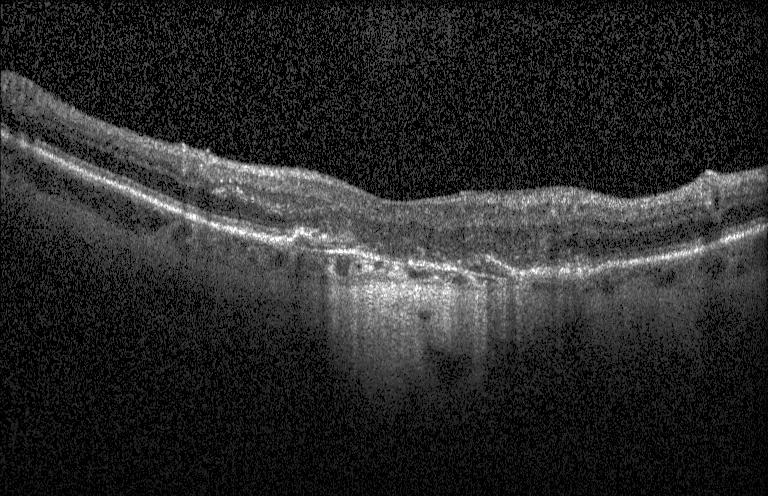

Retinal OCT B-scan. Centered on the fovea. Macular OCT: choroidal neovascularization (CNV).